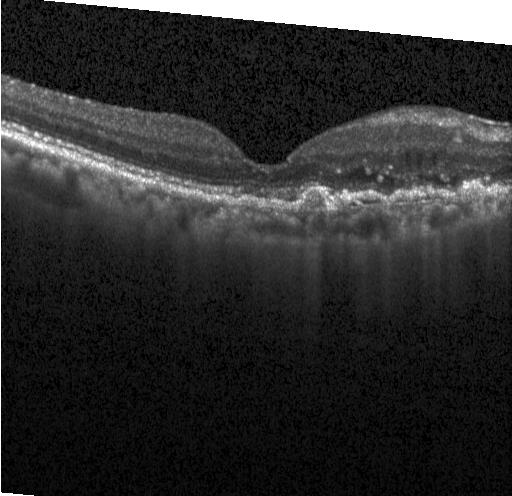 Diagnosis: choroidal neovascularization.